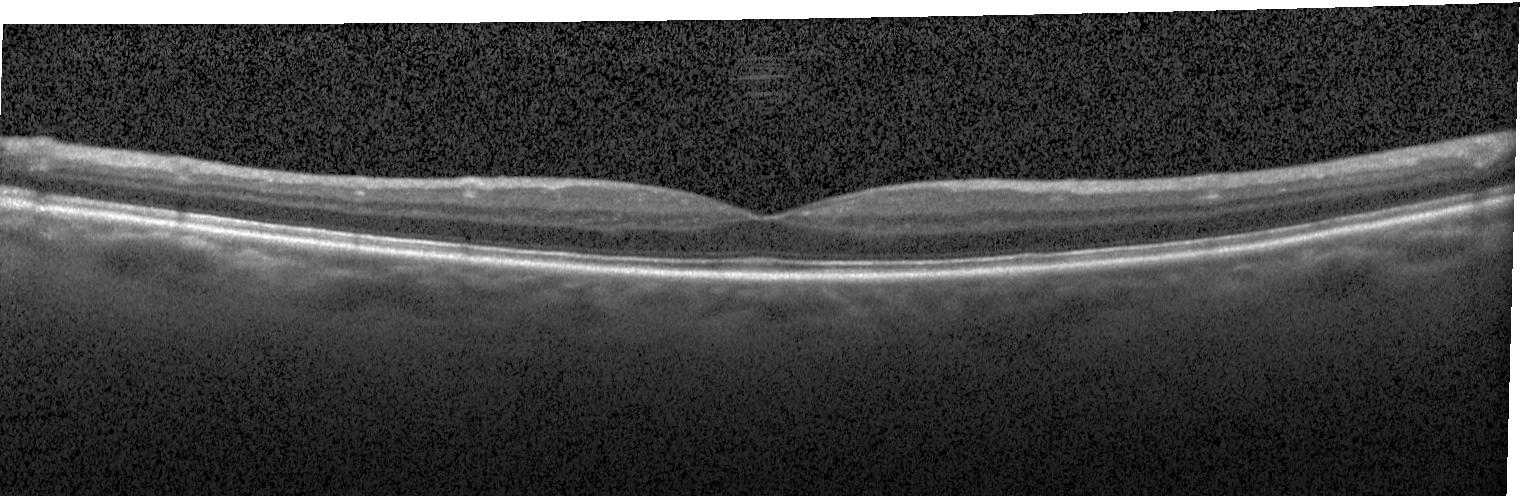

OCT B-scan. Heidelberg Spectralis OCT system. Through the macula. Spectral-domain OCT. This B-scan demonstrates no evidence of choroidal neovascularization, diabetic macular edema, or drusen.